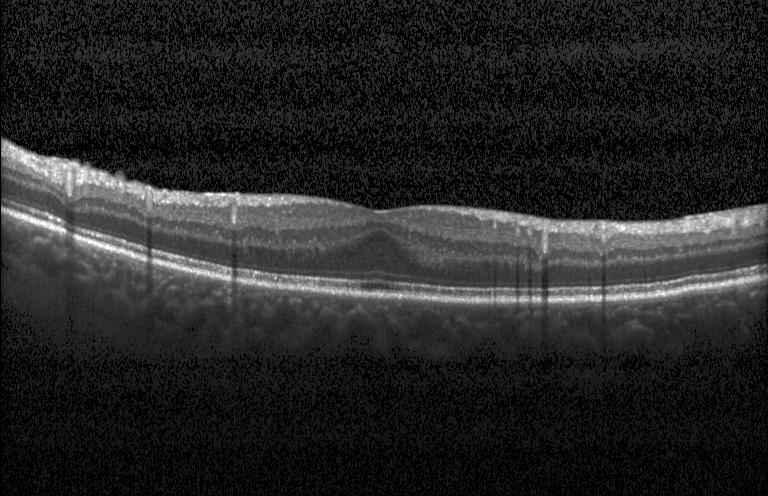
OCT B-scan — Macular OCT: neither choroidal neovascularization, diabetic macular edema, nor drusen.